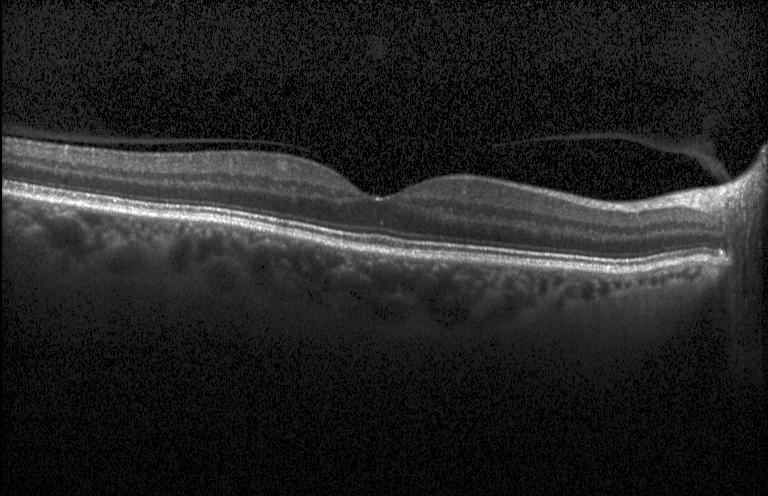 Acquired on a Heidelberg Spectralis. Horizontal scan through the fovea. Optical coherence tomography B-scan — Assessment: no CNV, DME, or drusen.